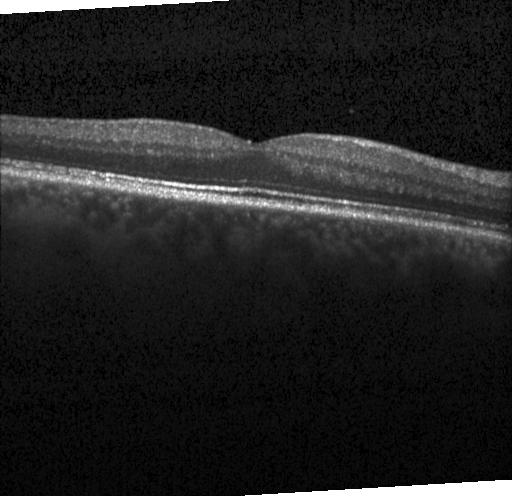

Optical coherence tomography B-scan; spectral-domain optical coherence tomography. The scan shows no choroidal neovascularization, diabetic macular edema, or drusen.